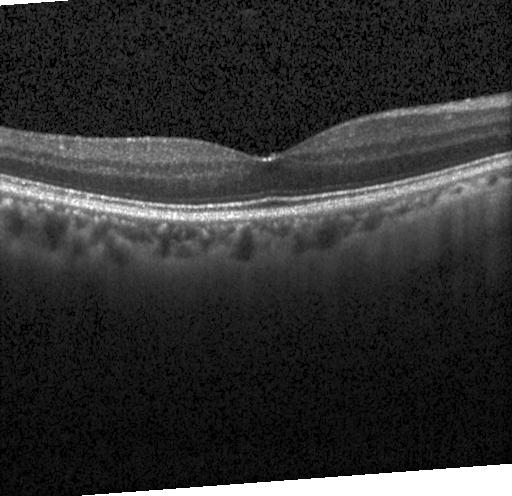 Through the macula, retinal OCT B-scan.
The scan shows no CNV, no DME, and no drusen.